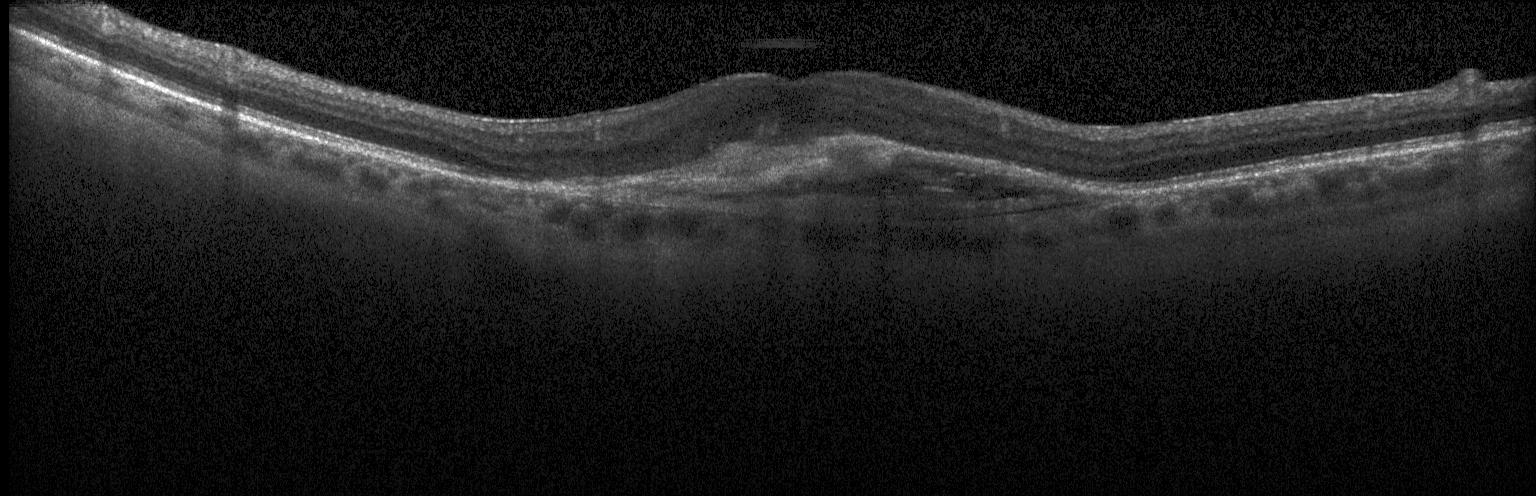

Diagnosis: choroidal neovascularization (CNV).